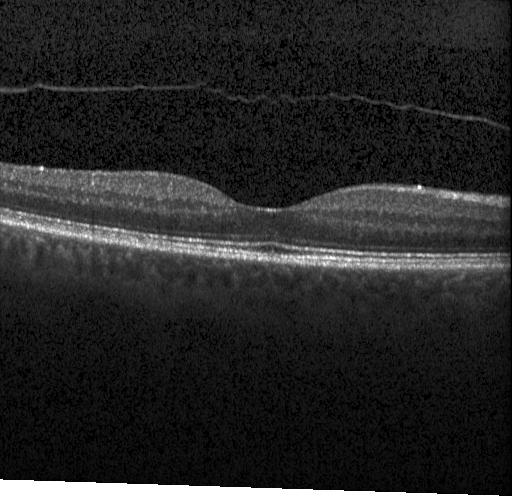
Assessment: neither choroidal neovascularization, diabetic macular edema, nor drusen.